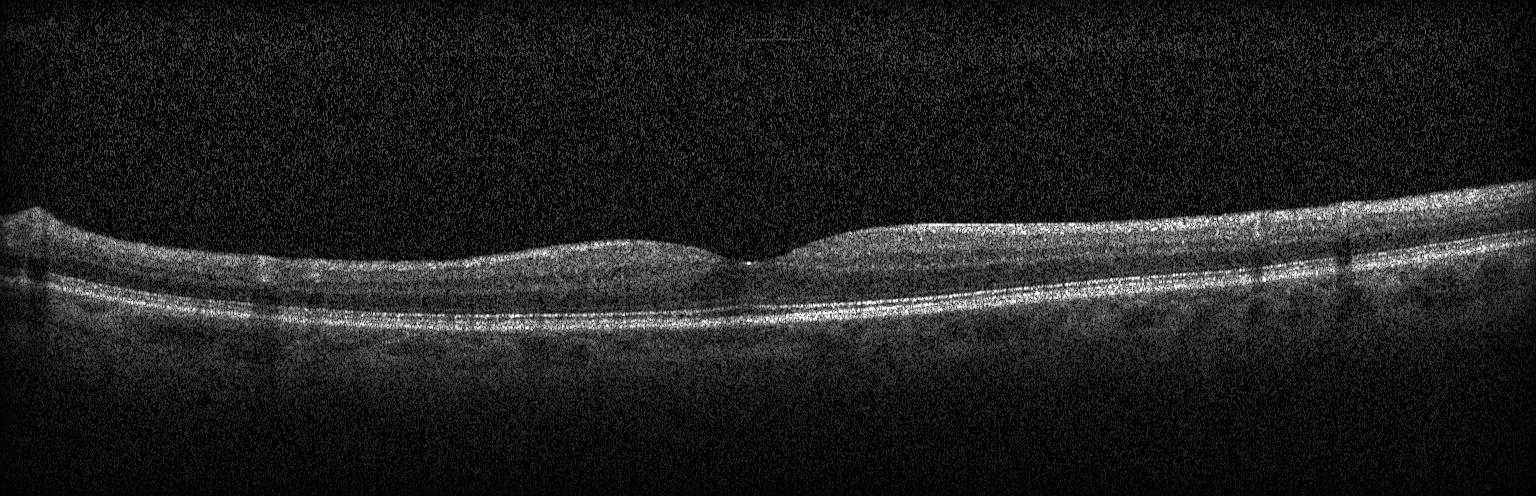
Spectral-domain OCT. Instrument: Heidelberg Spectralis. Optical coherence tomography B-scan
Dx: no CNV, DME, or drusen.